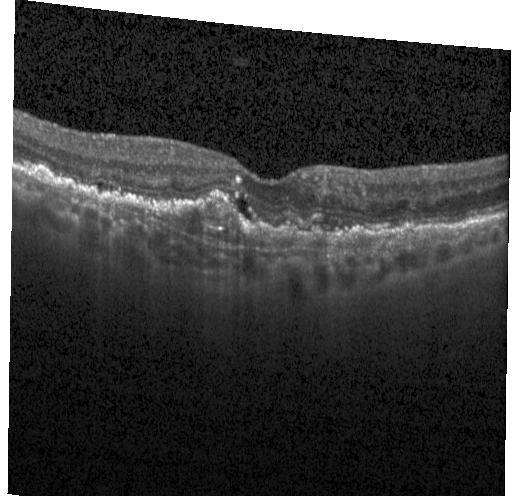
Macular OCT: choroidal neovascularization.